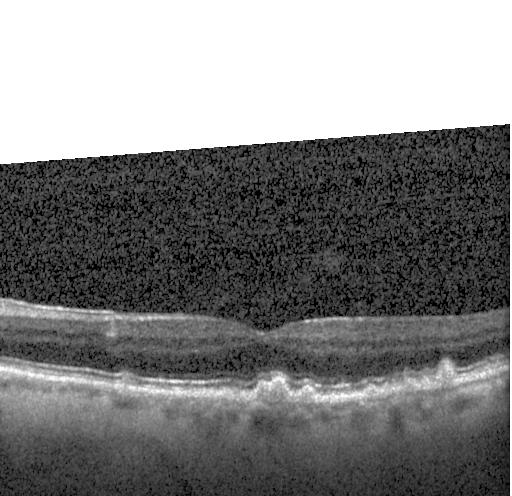
Macular OCT demonstrating sub-RPE drusenoid deposits.